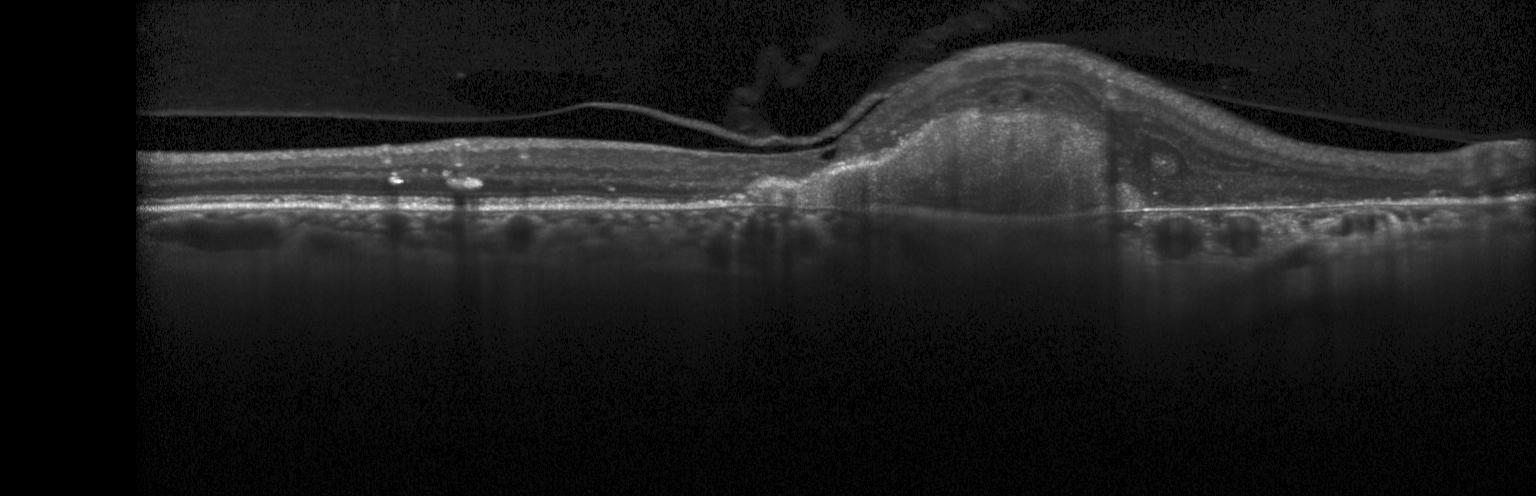 Assessment: a choroidal neovascular membrane.